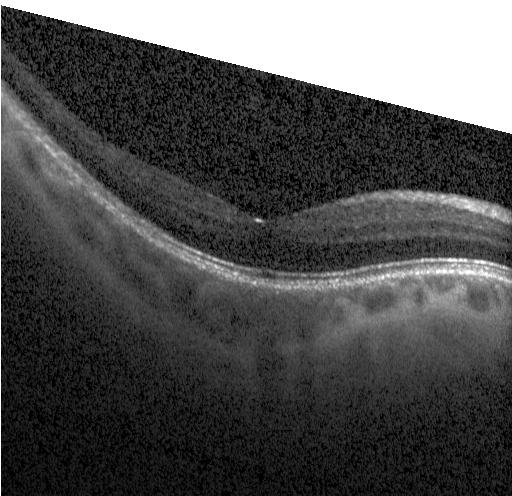
Heidelberg Spectralis OCT system · retinal OCT cross-section
The scan shows no choroidal neovascularization, diabetic macular edema, or drusen.